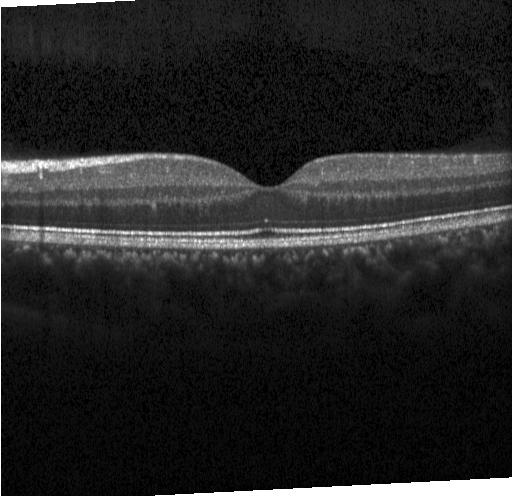 OCT B-scan · instrument: Heidelberg Spectralis · horizontal scan through the fovea · spectral-domain optical coherence tomography.
Finding: no choroidal neovascularization, no diabetic macular edema, and no drusen.